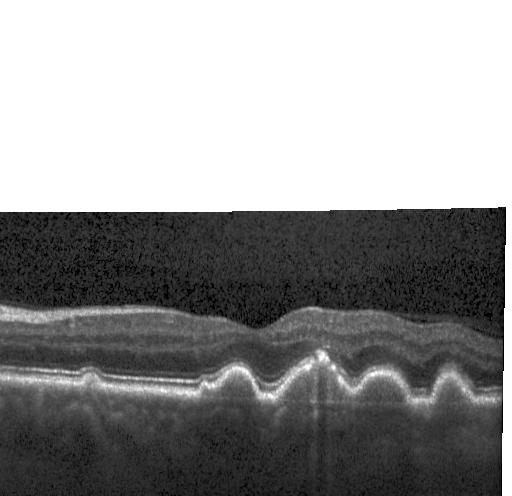
OCT B-scan. Macular scan. Acquired on a Heidelberg Spectralis.
Finding: multiple drusen.